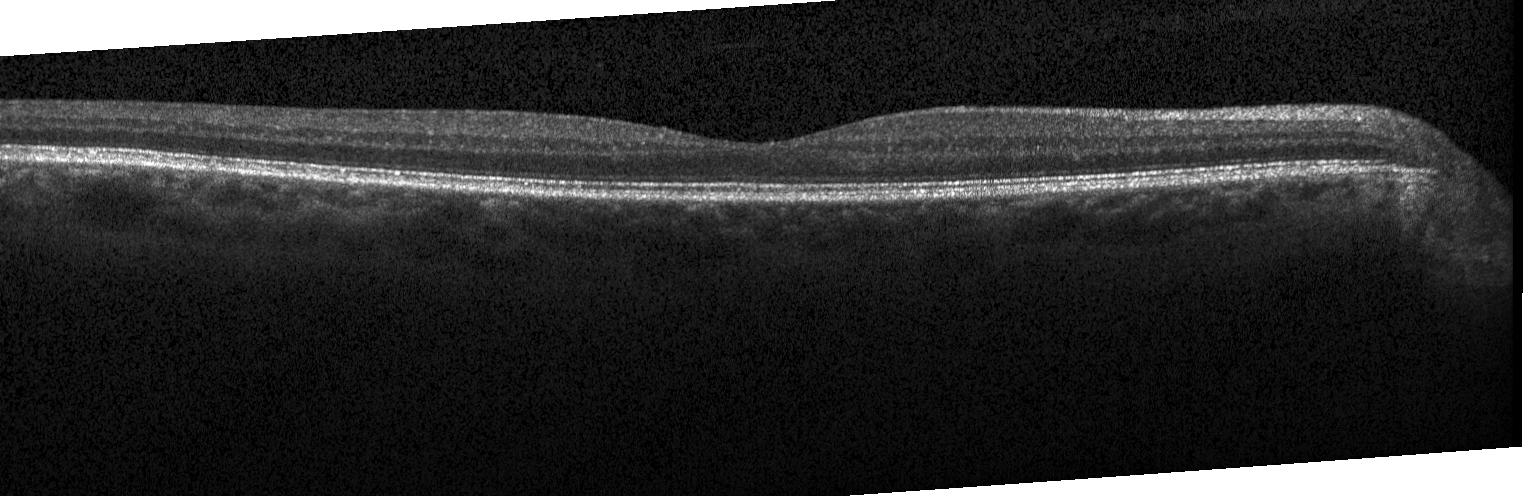

Retinal OCT B-scan; Heidelberg Spectralis; spectral-domain optical coherence tomography
Finding: no evidence of choroidal neovascularization, diabetic macular edema, or drusen.